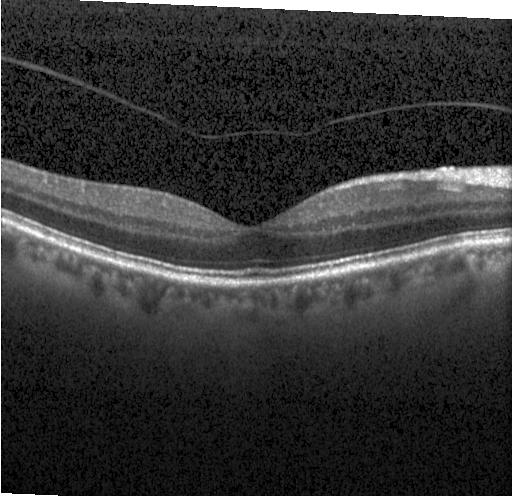 Acquired on a Heidelberg Spectralis · retinal OCT B-scan · spectral-domain OCT. Assessment: no choroidal neovascularization, diabetic macular edema, or drusen.